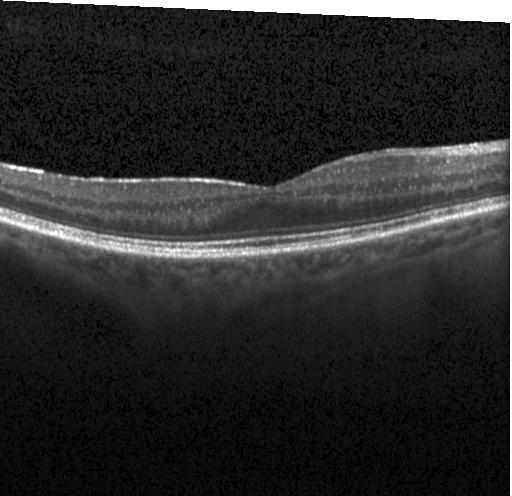

Impression: neither choroidal neovascularization, diabetic macular edema, nor drusen.